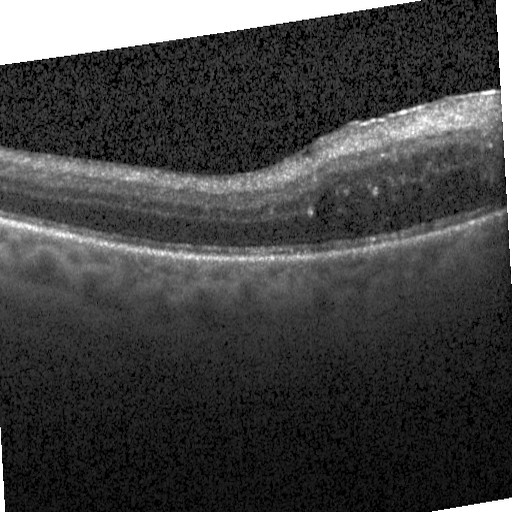

This B-scan demonstrates diabetic macular edema.